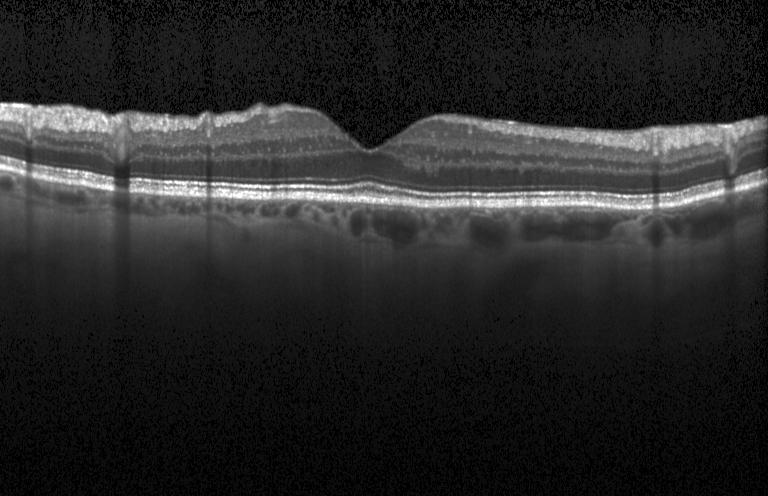
Retinal OCT B-scan, macular scan. Assessment: no choroidal neovascularization, no diabetic macular edema, and no drusen.